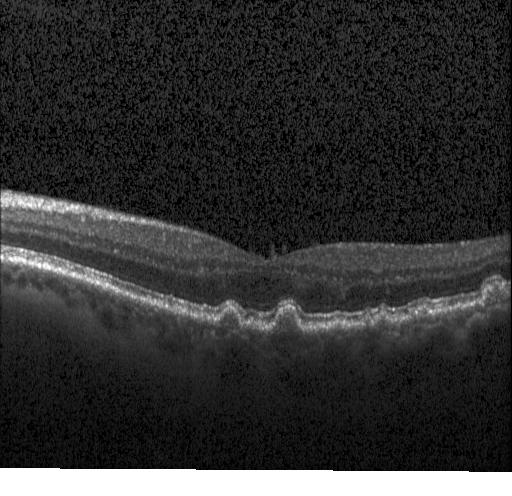
Dx: multiple drusen.